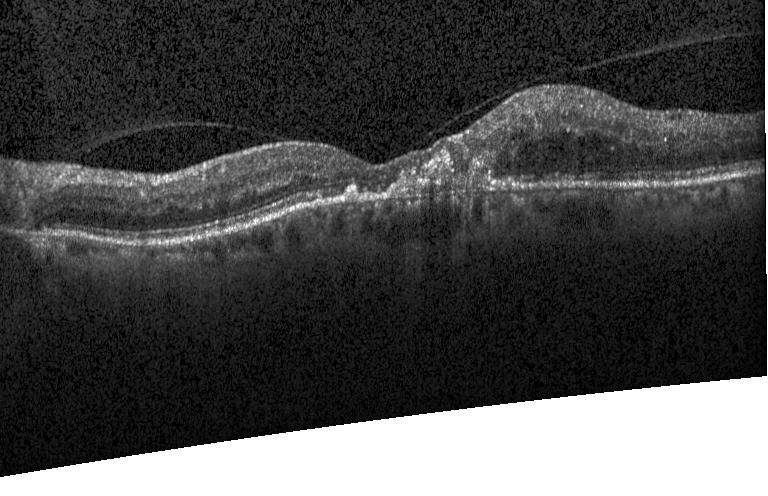

Optical coherence tomography scan. Spectral-domain OCT. This B-scan demonstrates CNV.